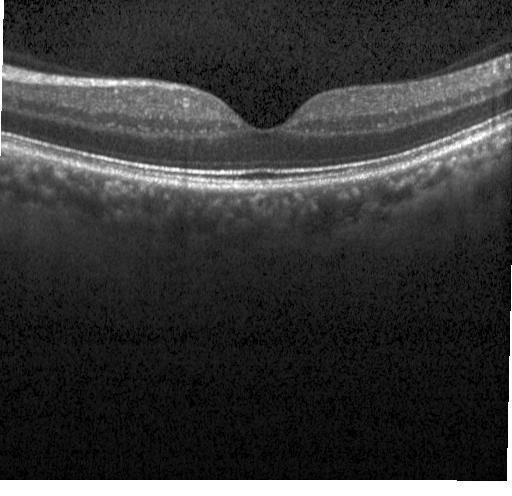
Impression: no CNV, no DME, and no drusen.